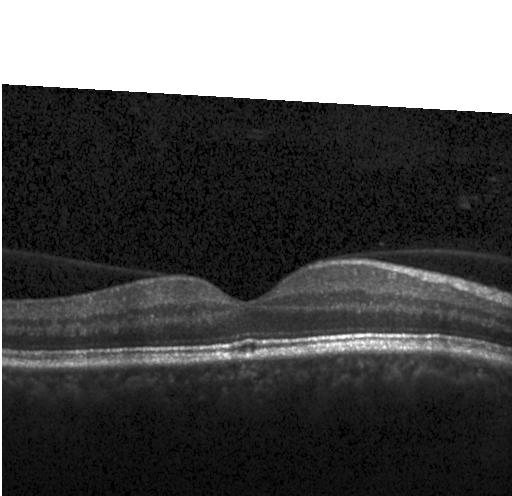 Finding: no choroidal neovascularization, no diabetic macular edema, and no drusen.